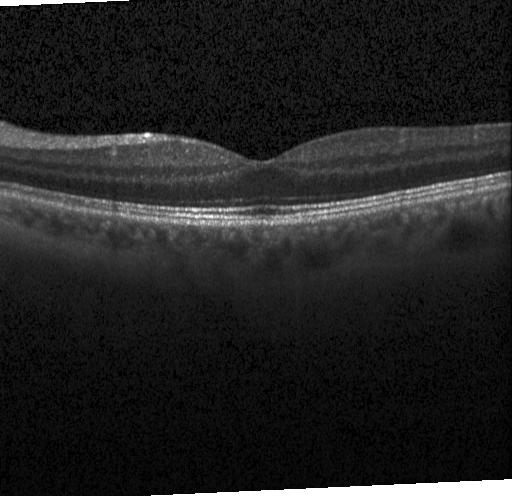

Fovea-centered · retinal OCT B-scan.
Diagnosis: neither choroidal neovascularization, diabetic macular edema, nor drusen.